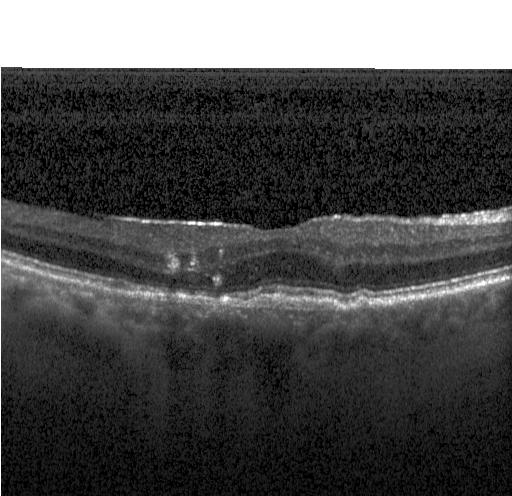 Diagnosis: CNV.